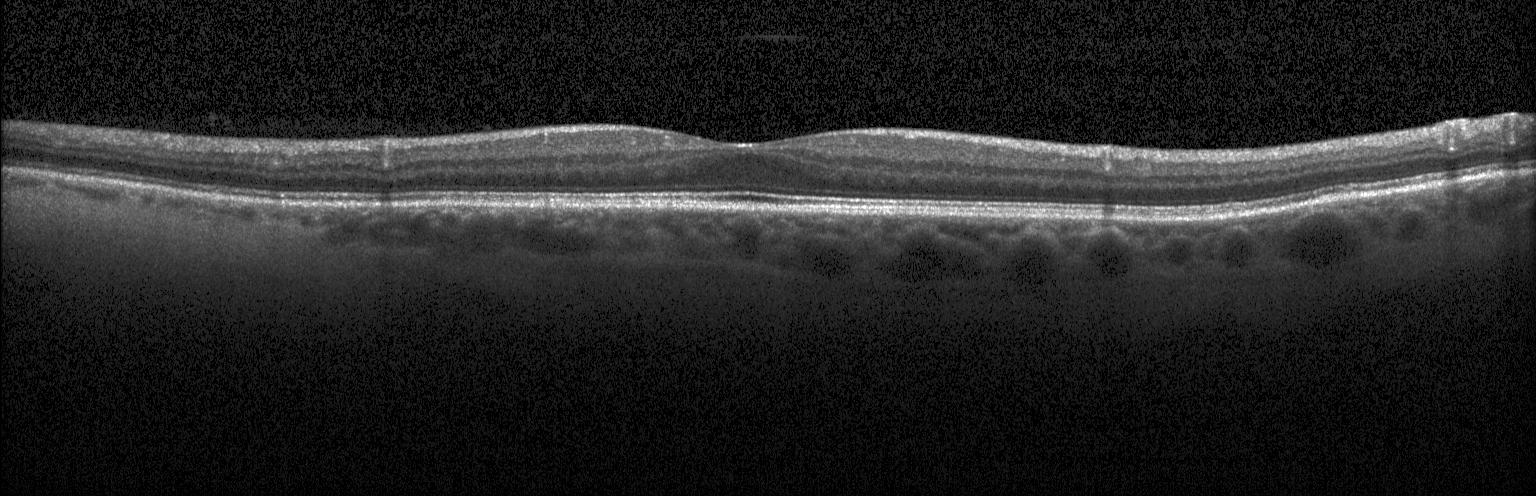 Retinal OCT cross-section; horizontal scan through the fovea.
Diagnosis: no choroidal neovascularization, diabetic macular edema, or drusen.